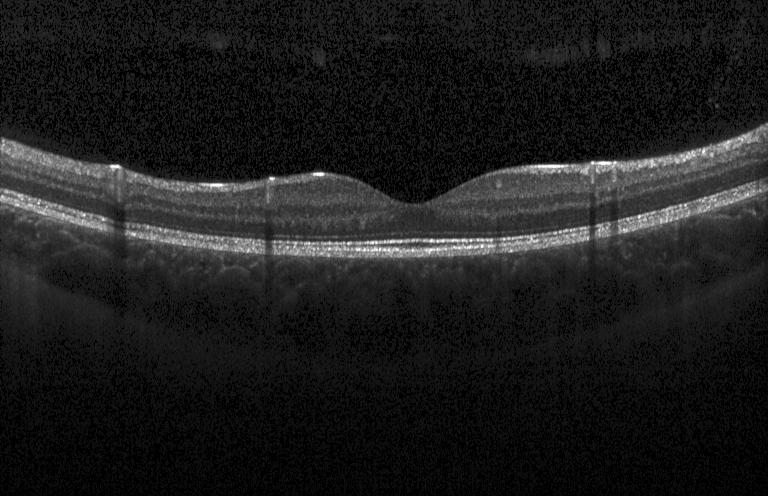 Heidelberg Spectralis · OCT B-scan. Diagnosis: no CNV, no DME, and no drusen.